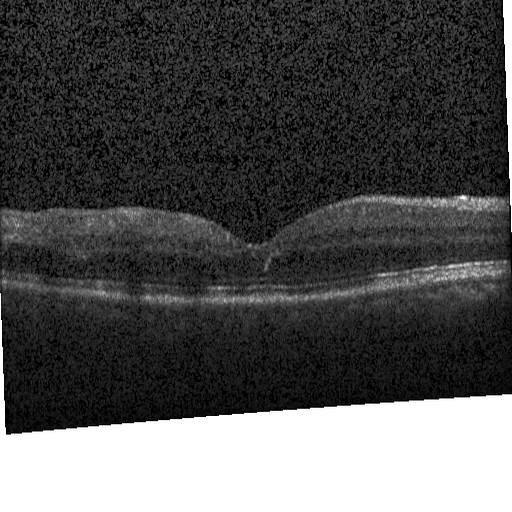 Assessment: DME.